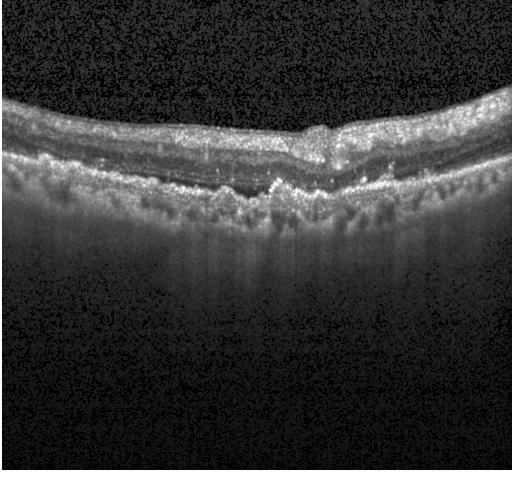
Retinal OCT B-scan; horizontal scan through the fovea. Macular OCT: choroidal neovascularization (CNV).